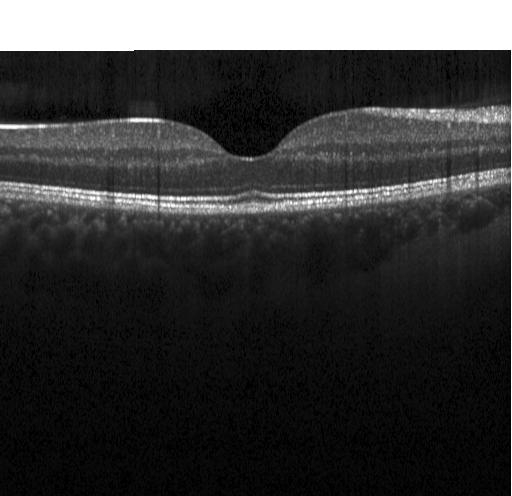 Impression: no choroidal neovascularization, no diabetic macular edema, and no drusen.